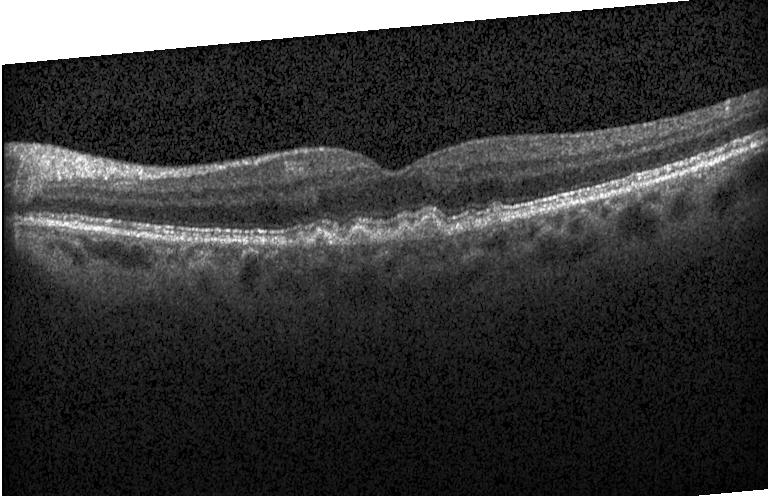
Impression: sub-RPE drusenoid deposits.